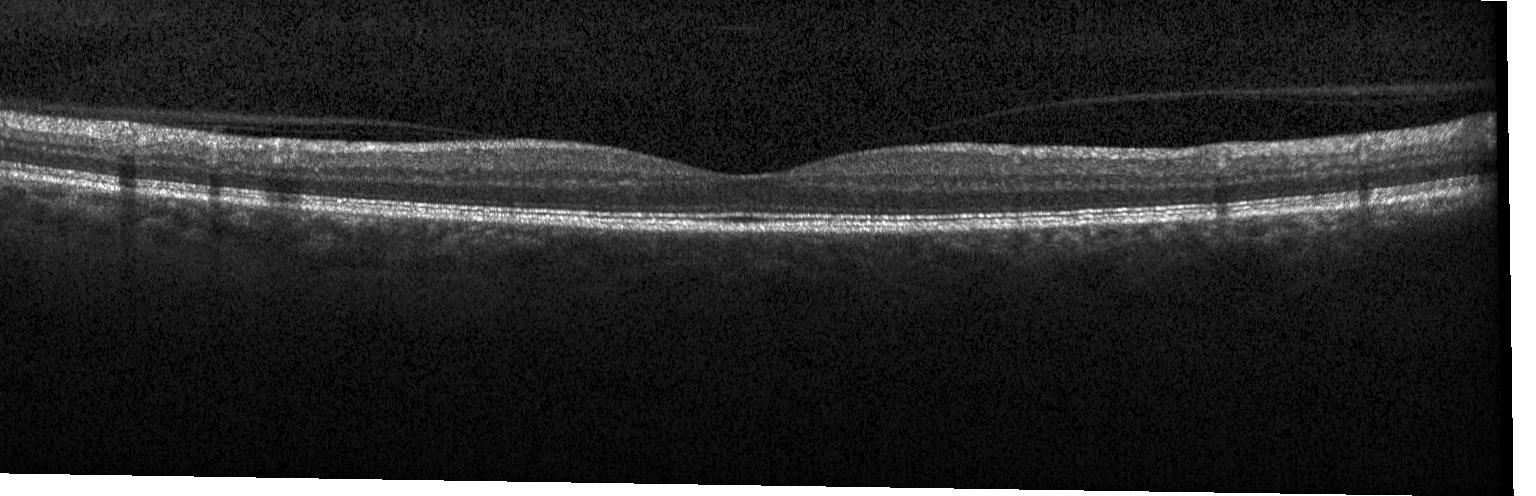
Impression: no CNV, no DME, and no drusen.